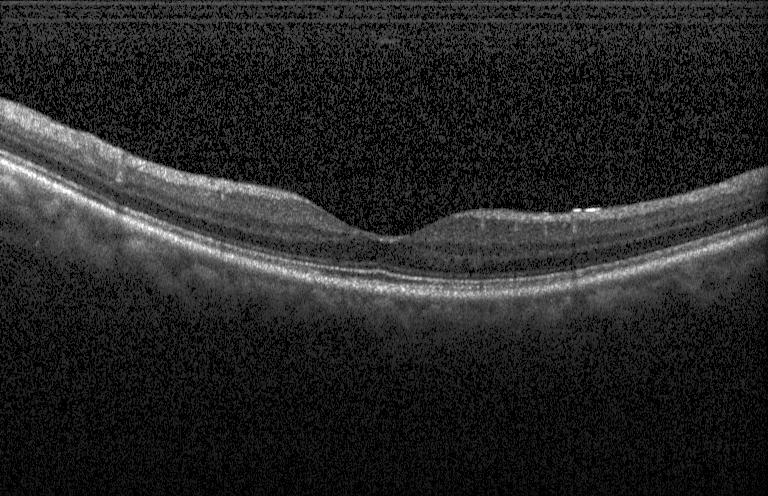
Finding: no choroidal neovascularization, no diabetic macular edema, and no drusen.